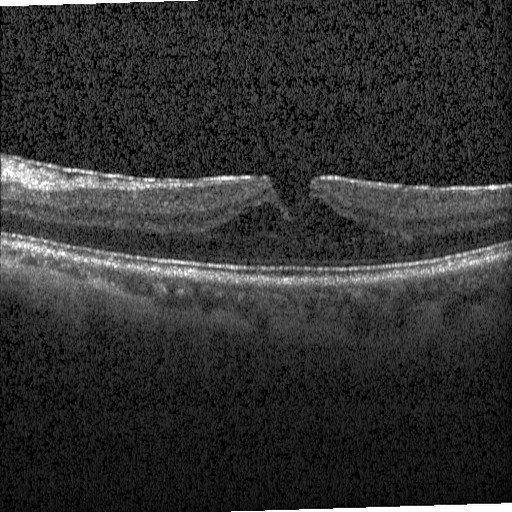
Horizontal scan through the fovea · Heidelberg Spectralis · optical coherence tomography scan · spectral-domain OCT. The scan shows DME.